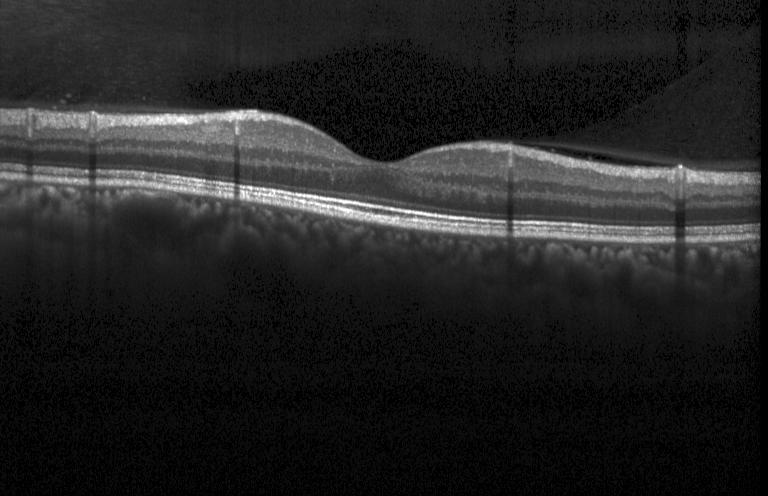 SD-OCT, optical coherence tomography B-scan, instrument: Heidelberg Spectralis, horizontal scan through the fovea — Diagnosis: no evidence of choroidal neovascularization, diabetic macular edema, or drusen.